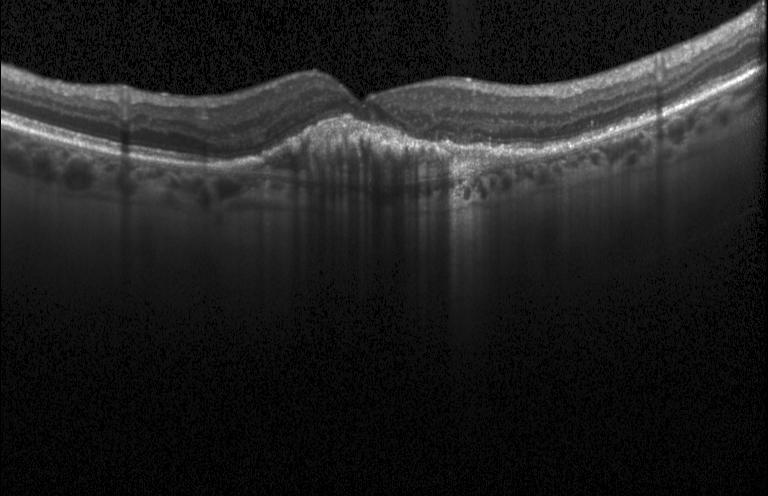 Optical coherence tomography scan; acquired on a Heidelberg Spectralis; fovea-centered; spectral-domain OCT
CNV.